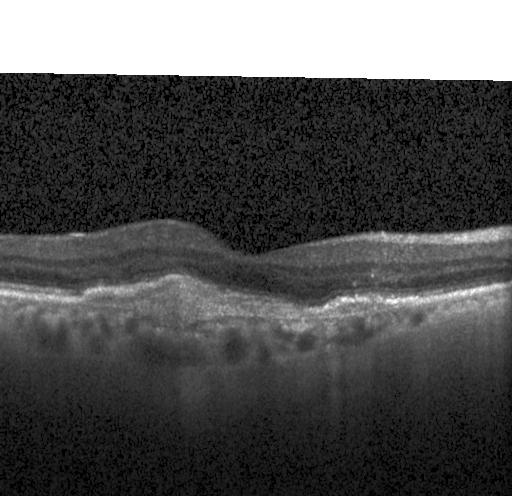
Heidelberg Spectralis · retinal OCT B-scan · SD-OCT. This B-scan demonstrates choroidal neovascularization.